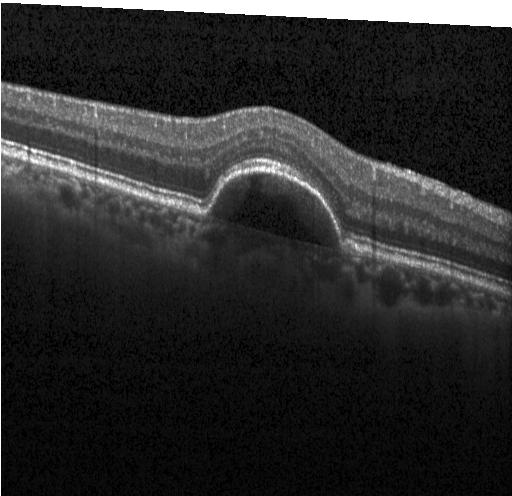
Retinal OCT cross-section; instrument: Heidelberg Spectralis. Finding: a choroidal neovascular membrane.